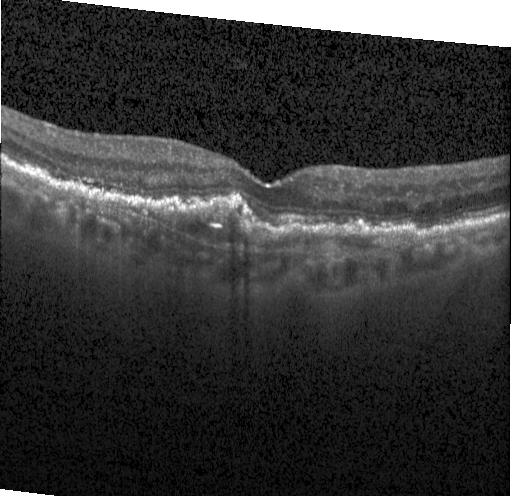 OCT line scan. Macular OCT: a choroidal neovascular membrane.